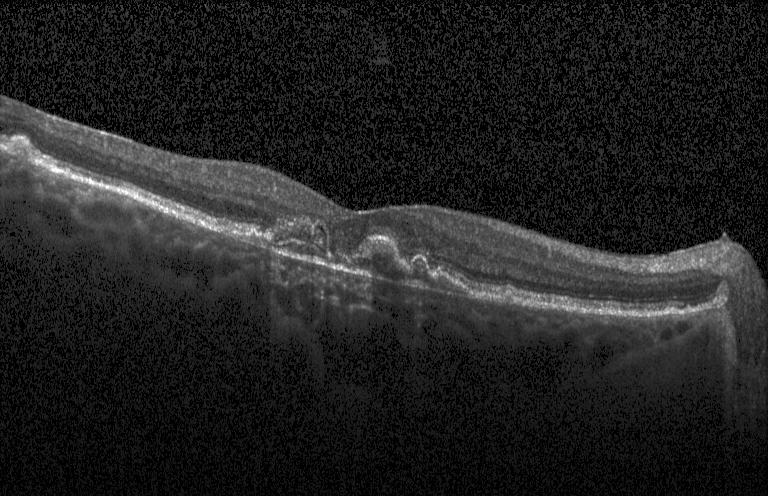

Diagnosis: a choroidal neovascular membrane.